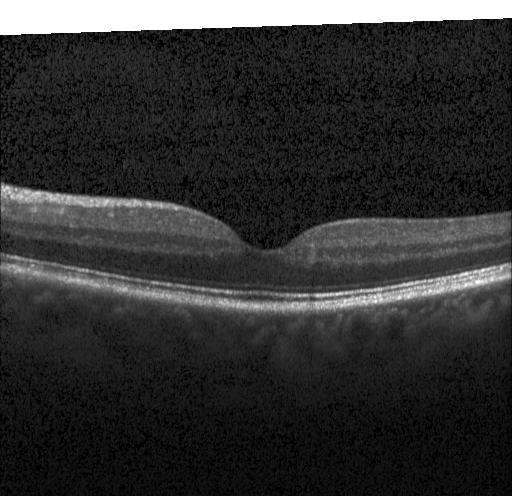

No choroidal neovascularization, diabetic macular edema, or drusen.